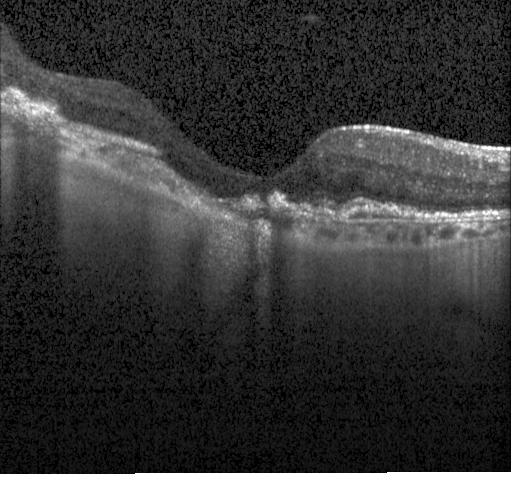
Heidelberg Spectralis, retinal OCT B-scan. Diagnosis: a choroidal neovascular membrane.